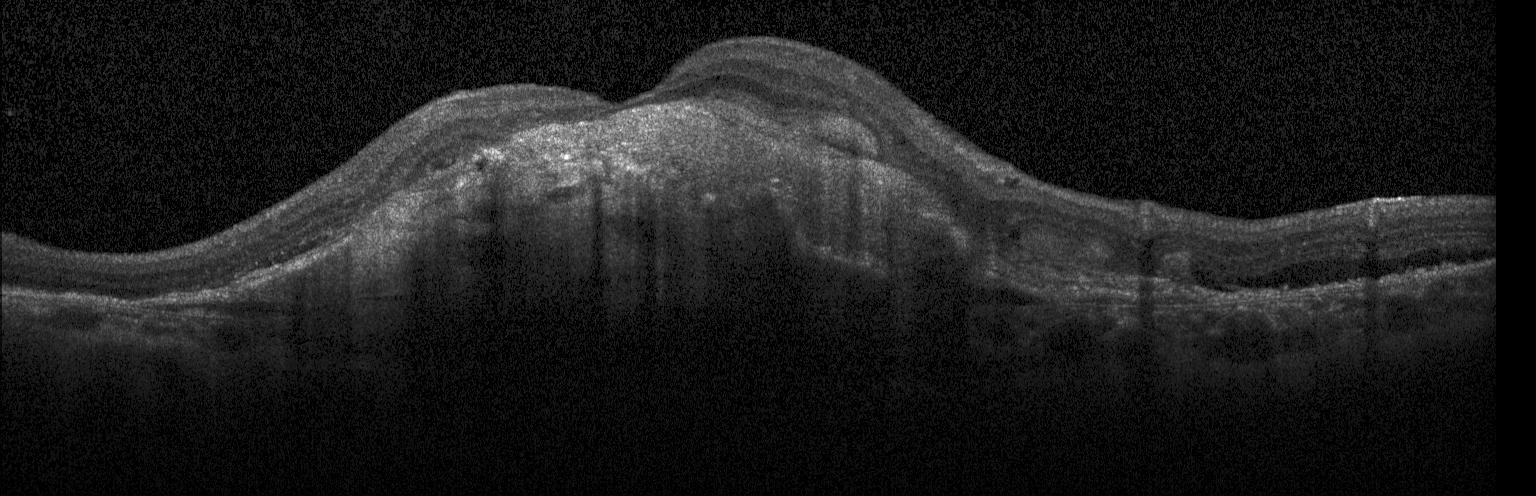

Instrument: Heidelberg Spectralis · OCT B-scan. Impression: a choroidal neovascular membrane.